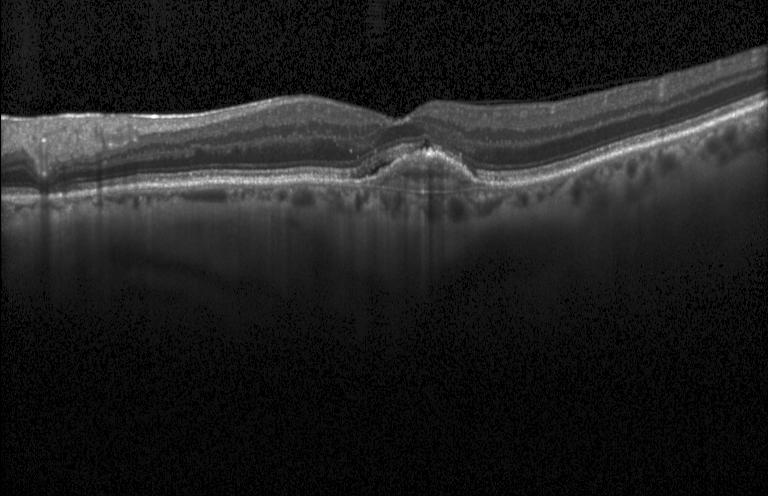

Macular OCT: choroidal neovascularization (CNV).